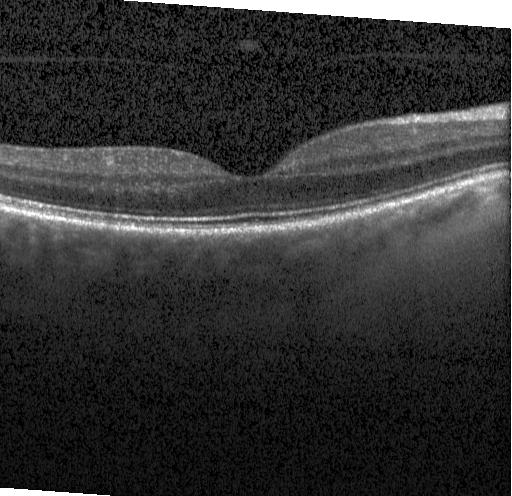
Optical coherence tomography scan — Diagnosis: no choroidal neovascularization, no diabetic macular edema, and no drusen.